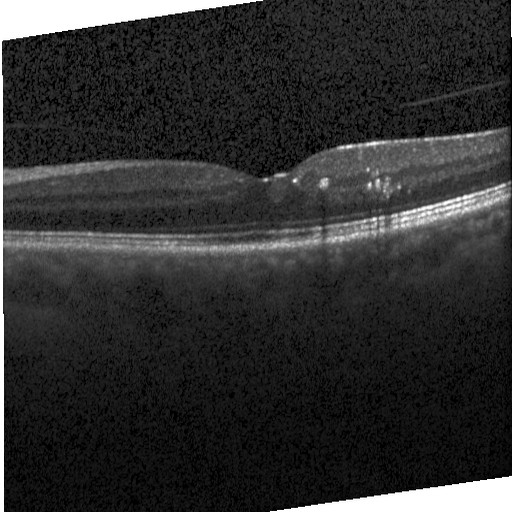

Through the macula · Heidelberg Spectralis · spectral-domain OCT · retinal OCT B-scan — Assessment: DME.